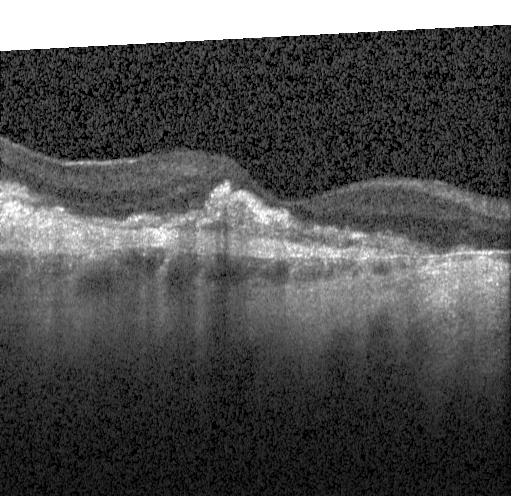 Macular OCT: a choroidal neovascular membrane.